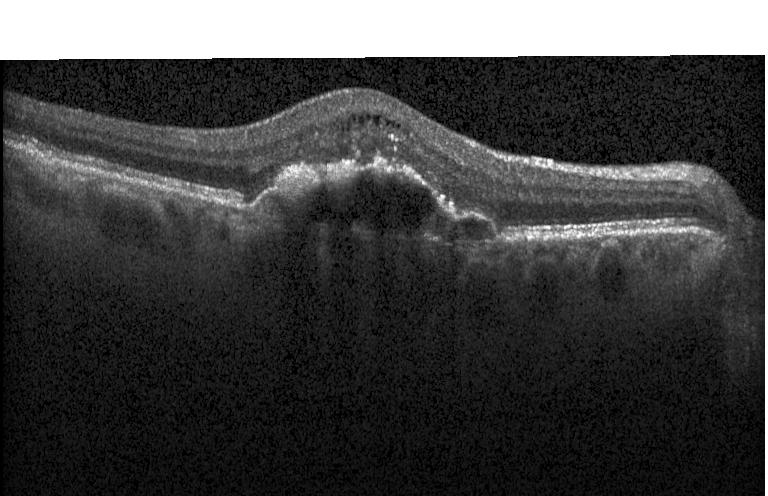
Diagnosis: a choroidal neovascular membrane.